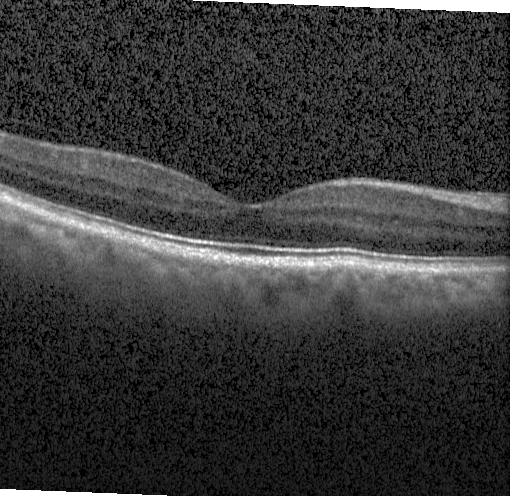
Heidelberg Spectralis; spectral-domain optical coherence tomography; retinal OCT B-scan; through the macula
Finding: neither choroidal neovascularization, diabetic macular edema, nor drusen.